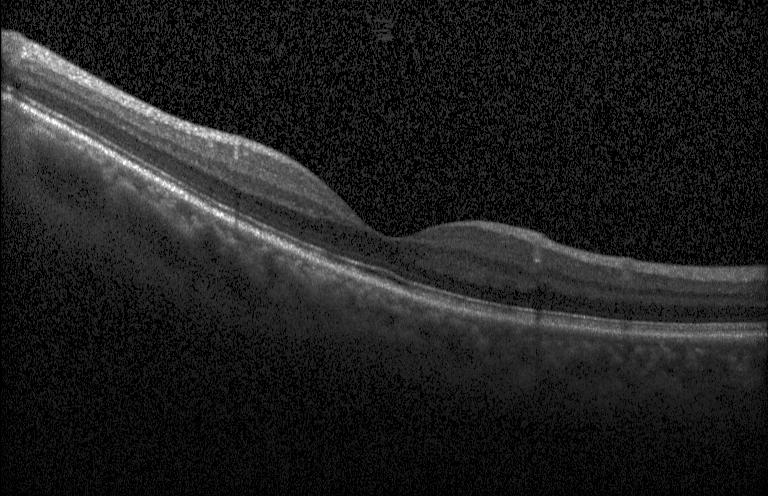

Impression: no CNV, no DME, and no drusen.